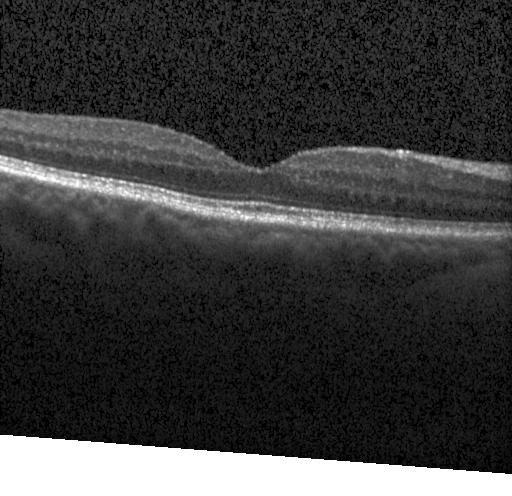
Optical coherence tomography B-scan. Horizontal scan through the fovea. Macular OCT: no choroidal neovascularization, diabetic macular edema, or drusen.